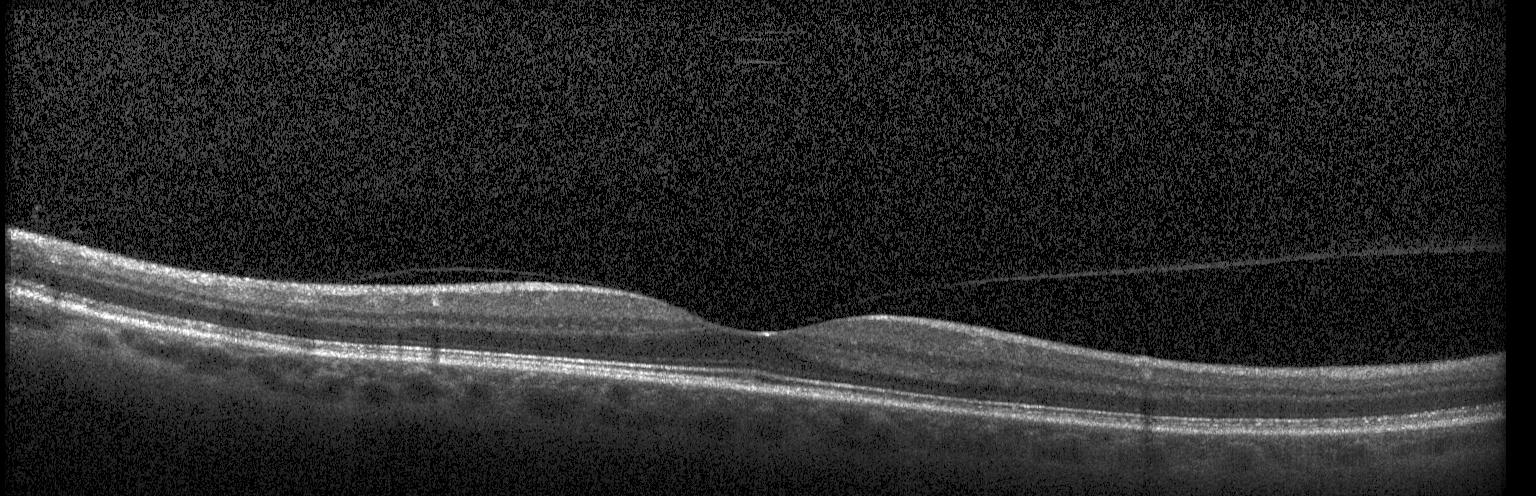 OCT B-scan
Dx: no CNV, no DME, and no drusen.